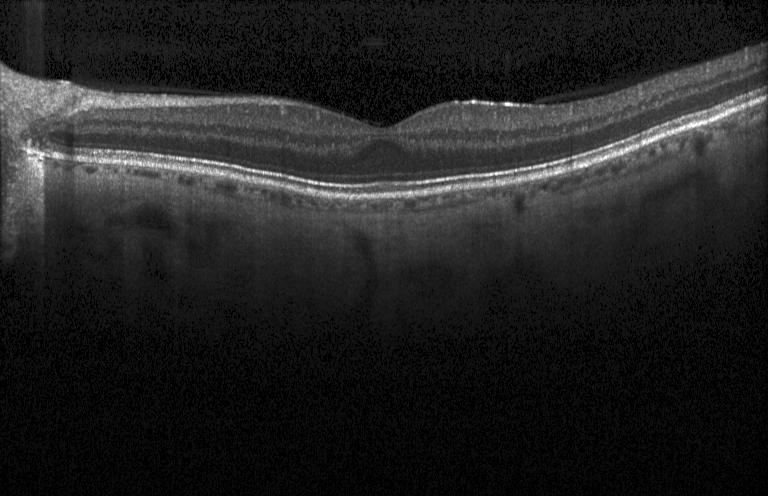
OCT B-scan. Dx: neither CNV, DME, nor drusen.